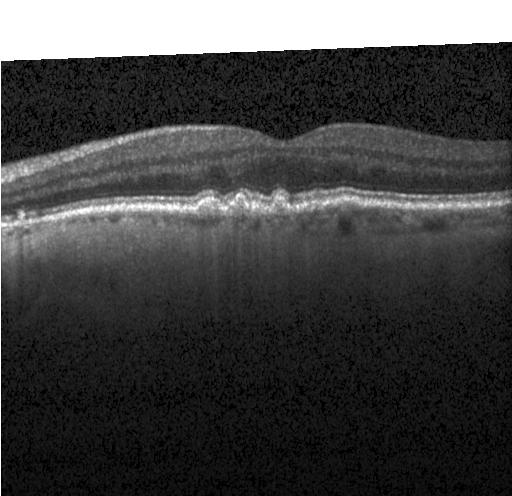 Optical coherence tomography B-scan. SD-OCT. Heidelberg Spectralis. Macular scan — This B-scan demonstrates sub-RPE drusenoid deposits.